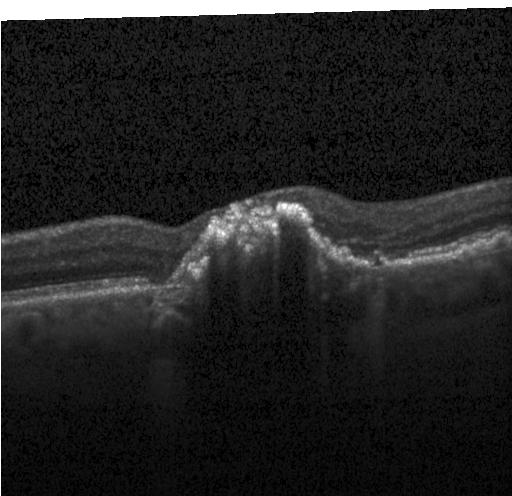 Macular scan, OCT B-scan, instrument: Heidelberg Spectralis. Impression: a choroidal neovascular membrane.